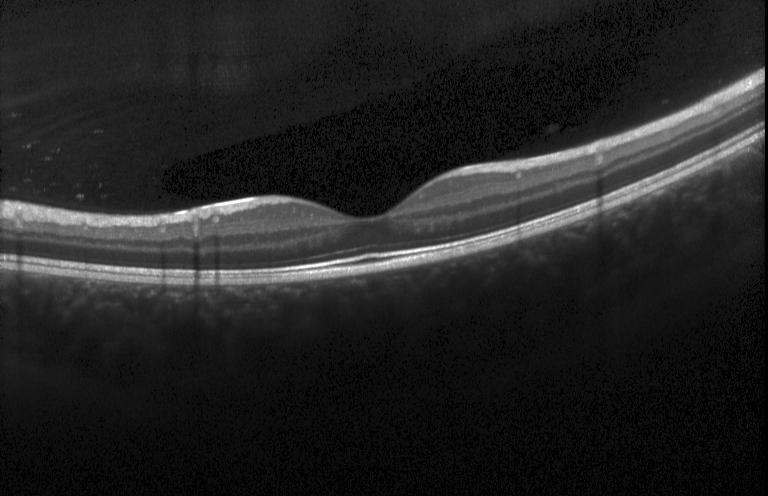 Retinal OCT cross-section · acquired on a Heidelberg Spectralis · SD-OCT · macular scan — Finding: neither CNV, DME, nor drusen.